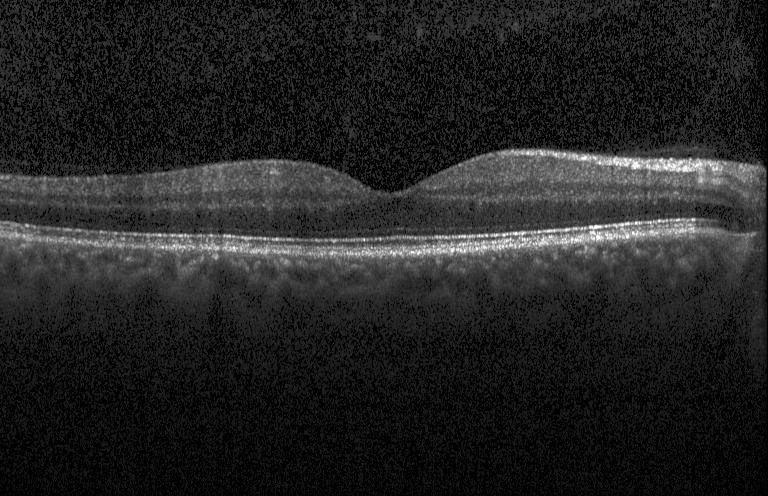 Impression: no choroidal neovascularization, no diabetic macular edema, and no drusen.